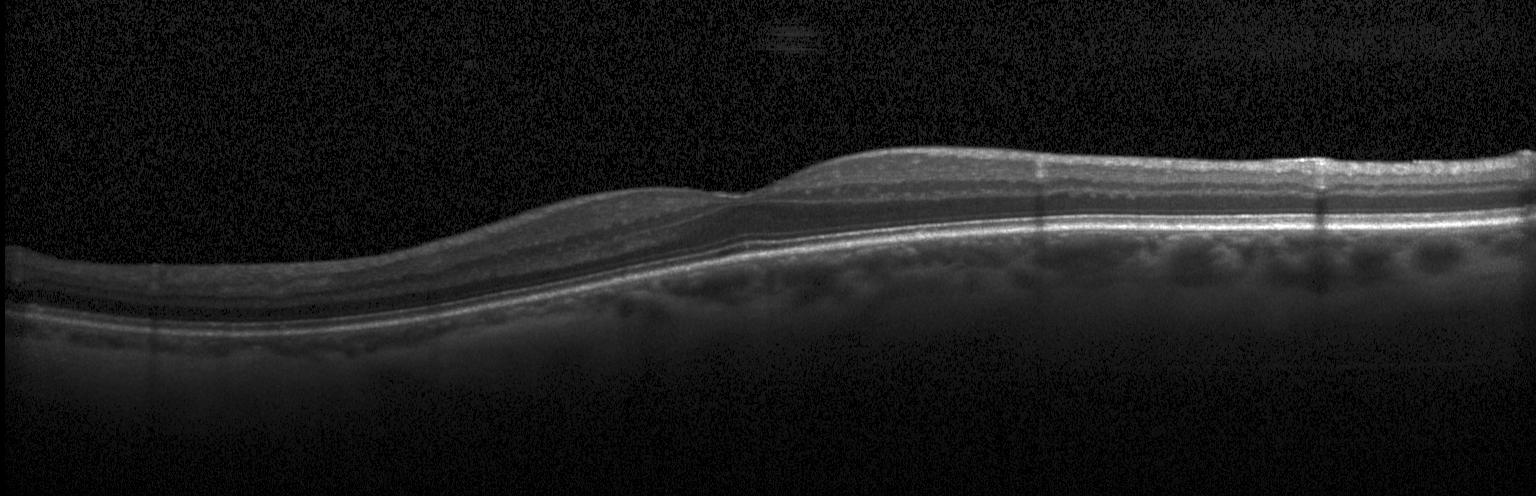

Impression: no CNV, DME, or drusen.